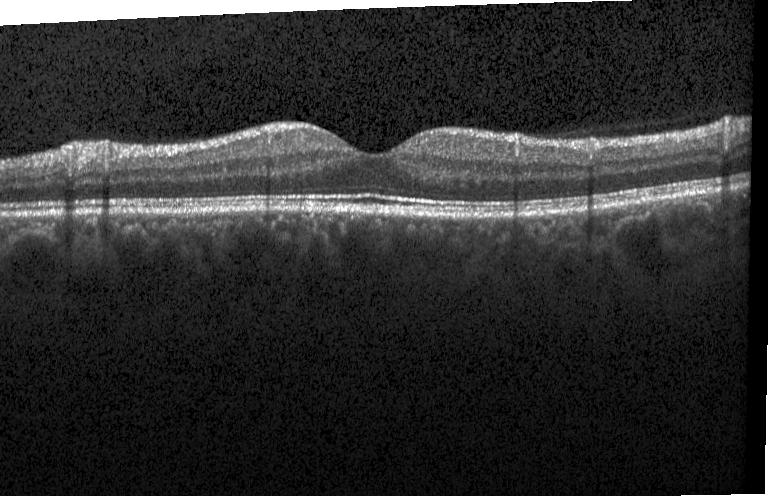

OCT B-scan showing neither CNV, DME, nor drusen.